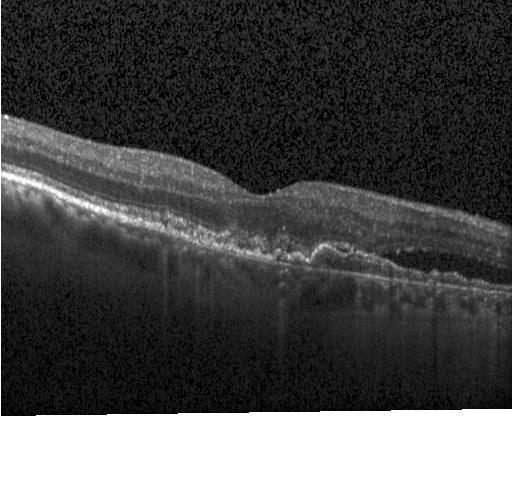
Optical coherence tomography B-scan · acquired on a Heidelberg Spectralis · spectral-domain optical coherence tomography. Impression: choroidal neovascularization.